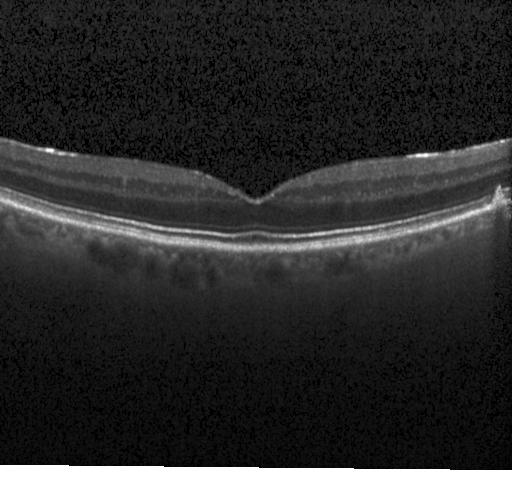
Dx: no CNV, DME, or drusen.